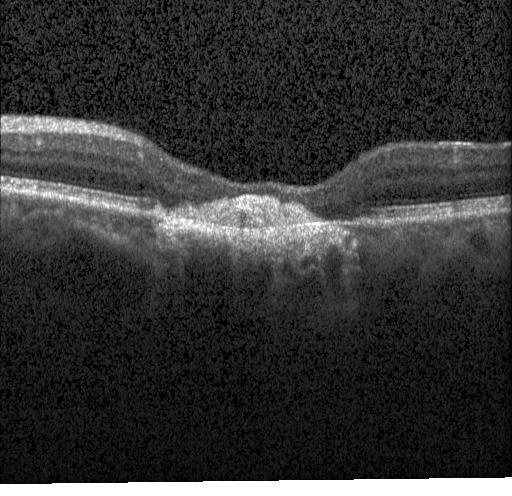 OCT line scan. Impression: a choroidal neovascular membrane.